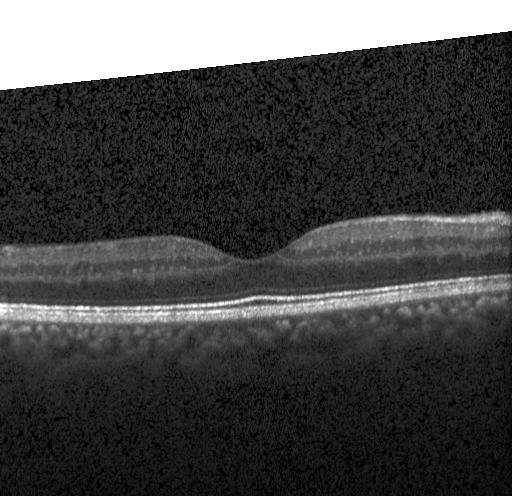

Optical coherence tomography scan — Impression: neither CNV, DME, nor drusen.